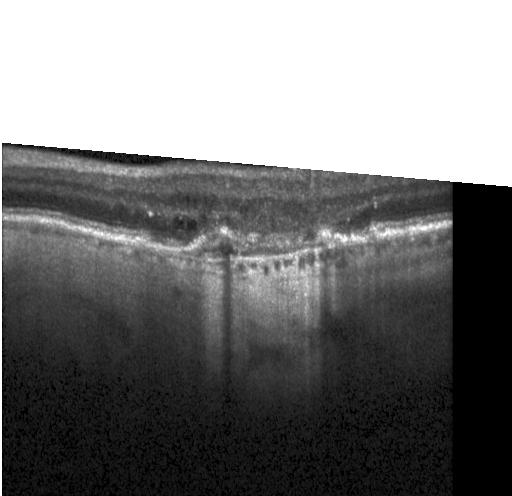 SD-OCT. Horizontal scan through the fovea. Retinal OCT cross-section. Acquired on a Heidelberg Spectralis
Impression: choroidal neovascularization.